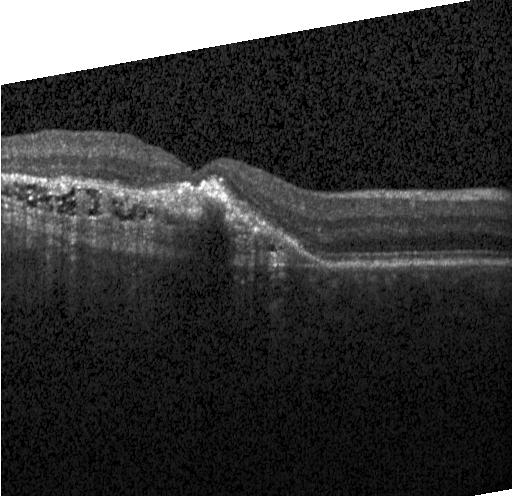 Through the macula; spectral-domain optical coherence tomography; optical coherence tomography scan.
The scan shows a choroidal neovascular membrane.